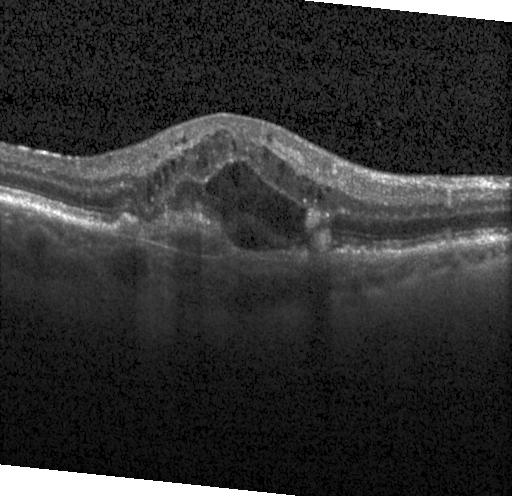

Macular scan; retinal OCT cross-section; spectral-domain optical coherence tomography; Heidelberg Spectralis OCT system — Diagnosis: choroidal neovascularization (CNV).